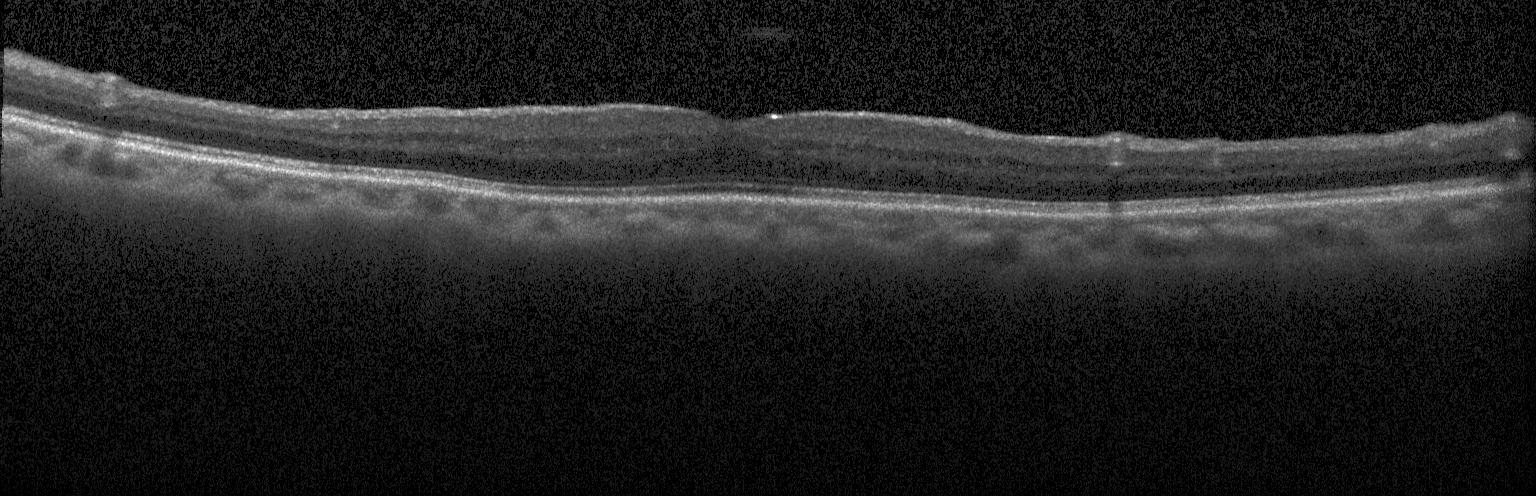

Retinal OCT B-scan; Heidelberg Spectralis; spectral-domain OCT.
Finding: no CNV, no DME, and no drusen.